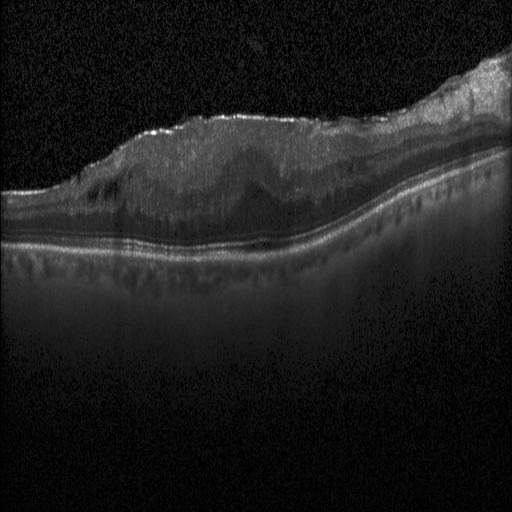
OCT finding: diabetic macular edema.